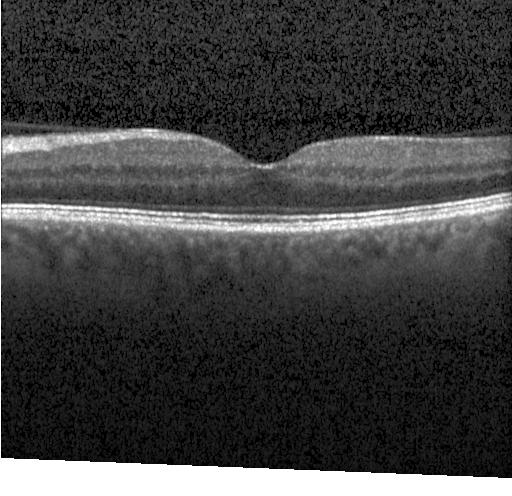 Retinal OCT B-scan, instrument: Heidelberg Spectralis, fovea-centered, spectral-domain optical coherence tomography.
Neither choroidal neovascularization, diabetic macular edema, nor drusen.